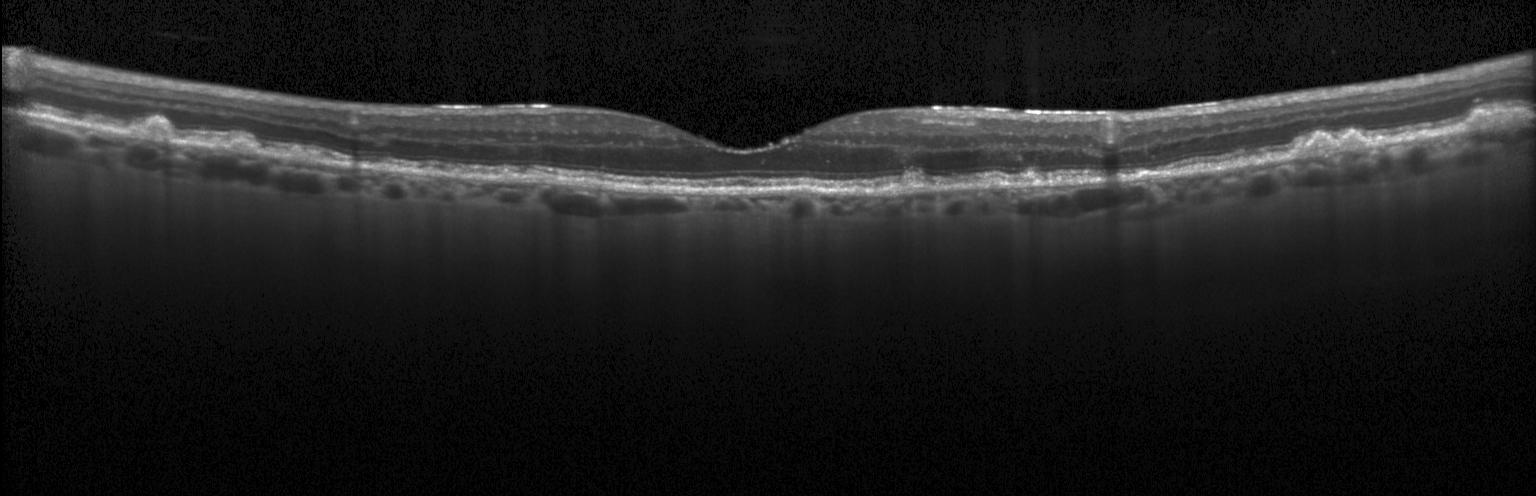

Retinal OCT B-scan. Acquired on a Heidelberg Spectralis. Fovea-centered.
Finding: drusen.